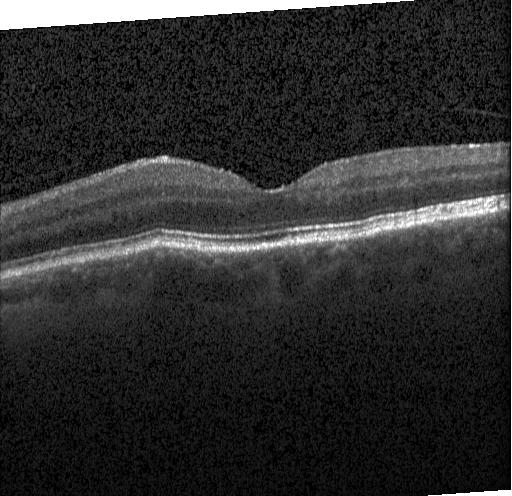 Diagnosis: no choroidal neovascularization, diabetic macular edema, or drusen.